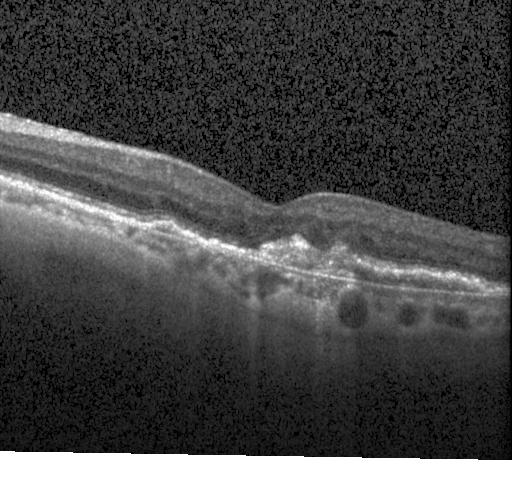

Optical coherence tomography B-scan. SD-OCT. Acquired on a Heidelberg Spectralis. Horizontal scan through the fovea — Finding: a choroidal neovascular membrane.